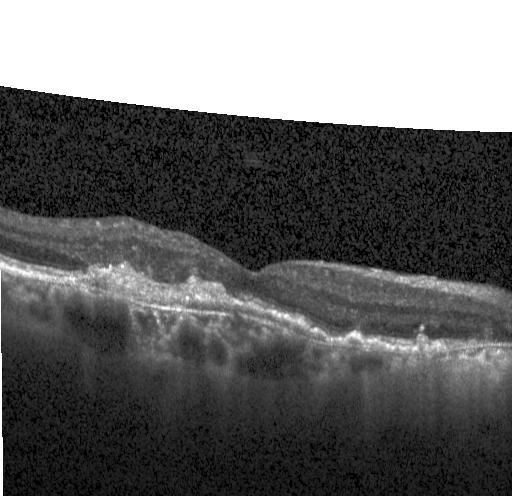
Finding: choroidal neovascularization (CNV).